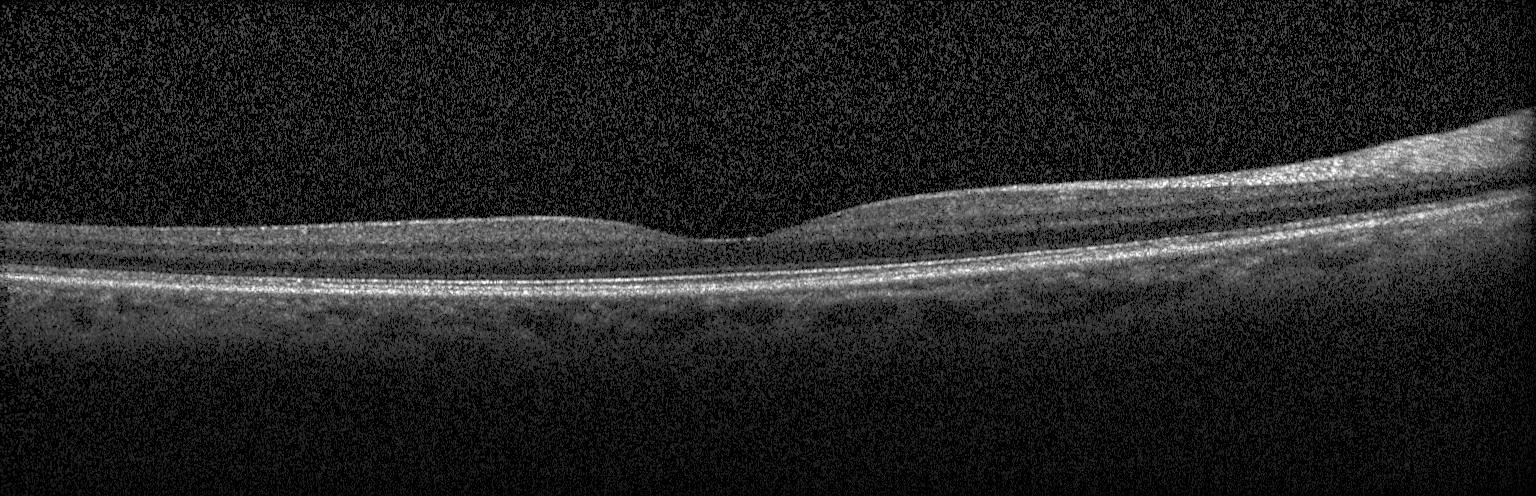 Finding: neither CNV, DME, nor drusen.